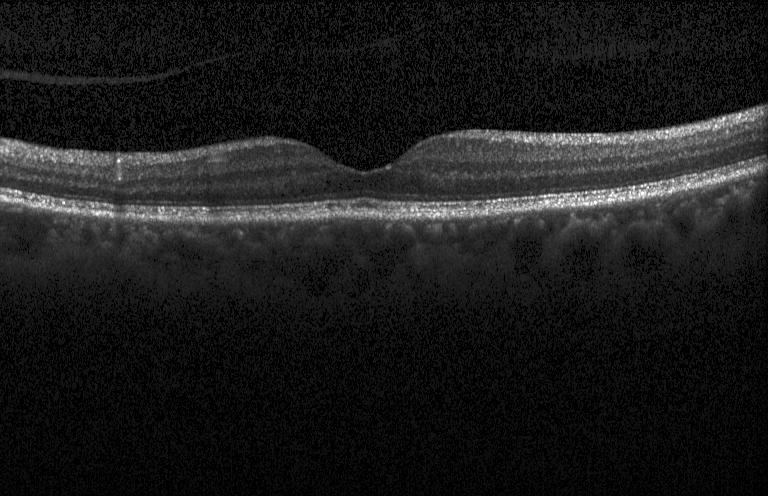

Macular OCT demonstrating no CNV, DME, or drusen.